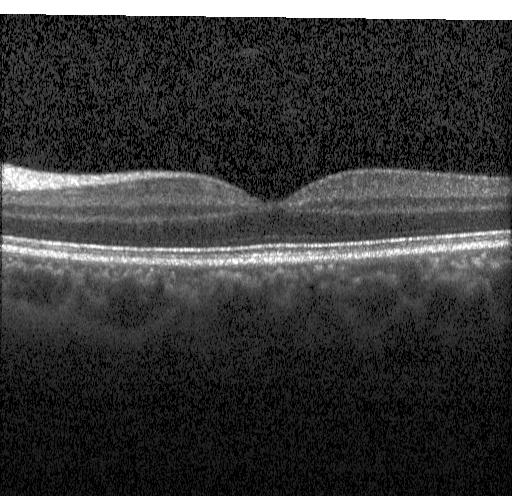

OCT line scan
Impression: neither choroidal neovascularization, diabetic macular edema, nor drusen.